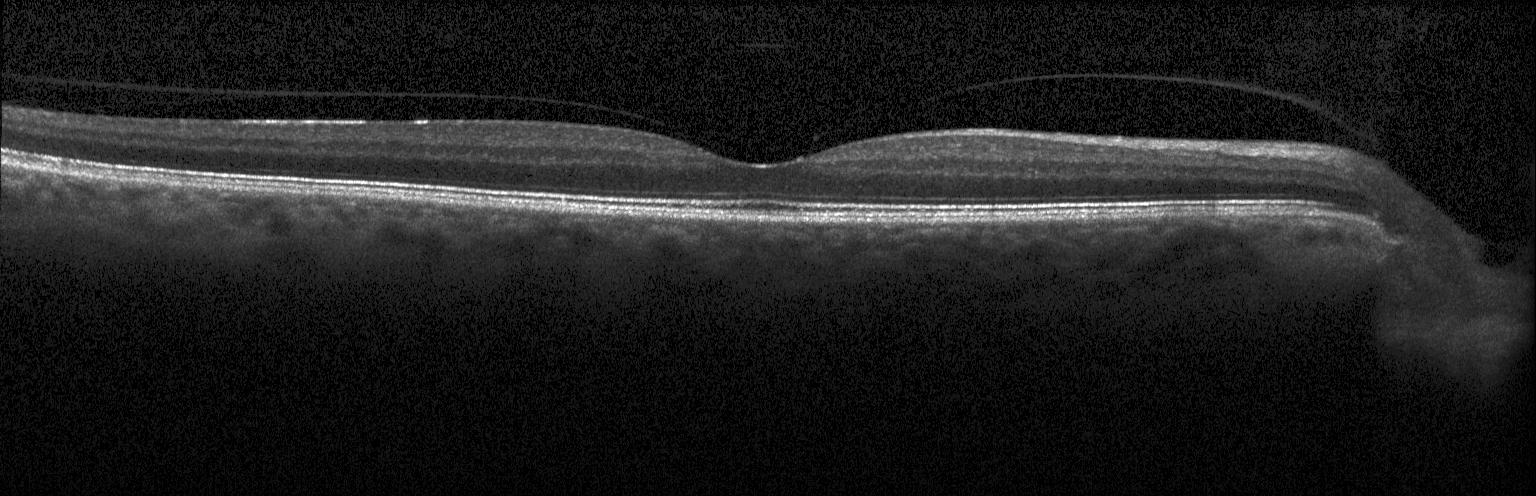
Diagnosis: no CNV, no DME, and no drusen.